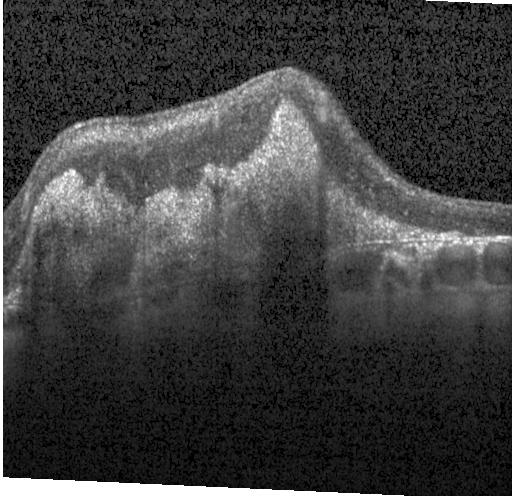

Impression: choroidal neovascularization.